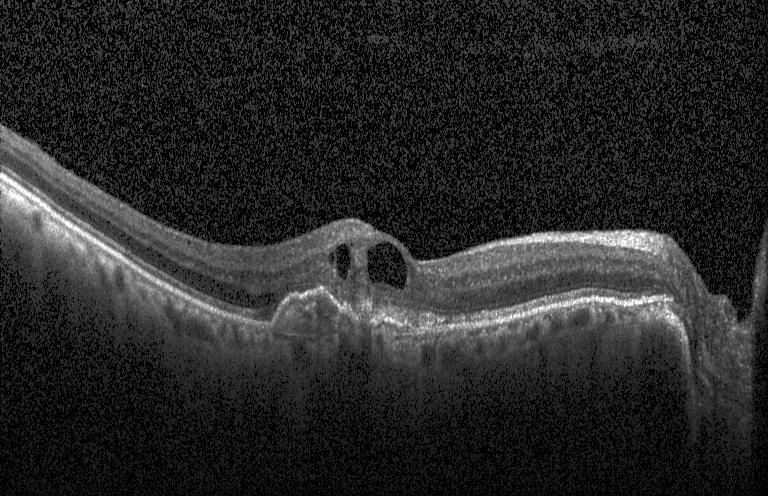 OCT B-scan. Finding: choroidal neovascularization.